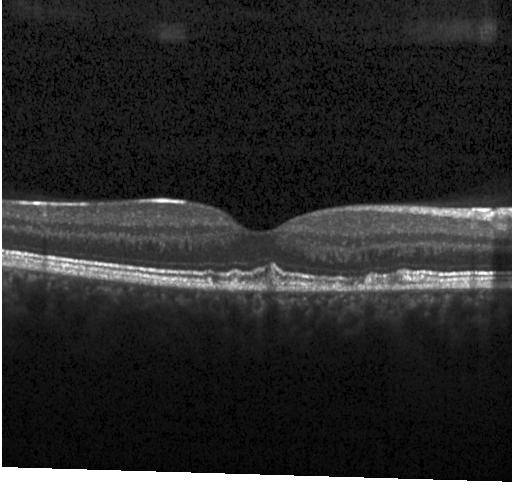

Finding: multiple drusen.